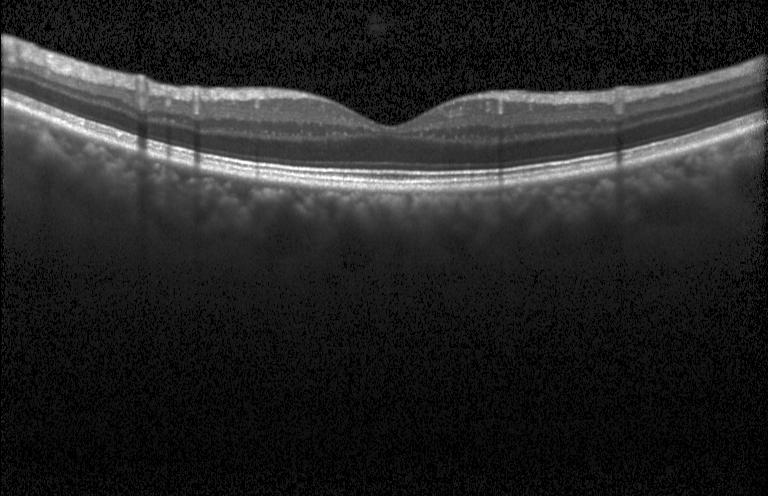 Impression: no evidence of choroidal neovascularization, diabetic macular edema, or drusen.